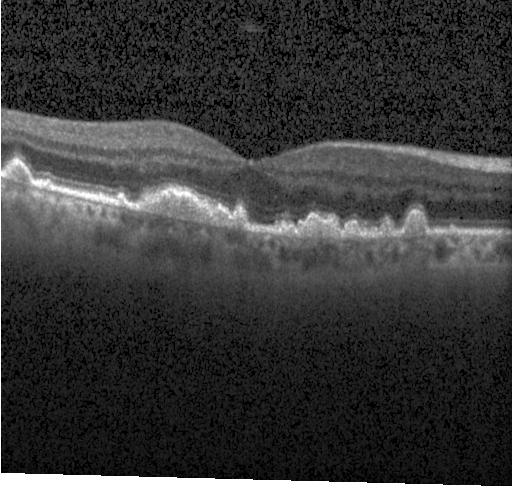 Heidelberg Spectralis · optical coherence tomography scan.
Diagnosis: sub-RPE drusenoid deposits.